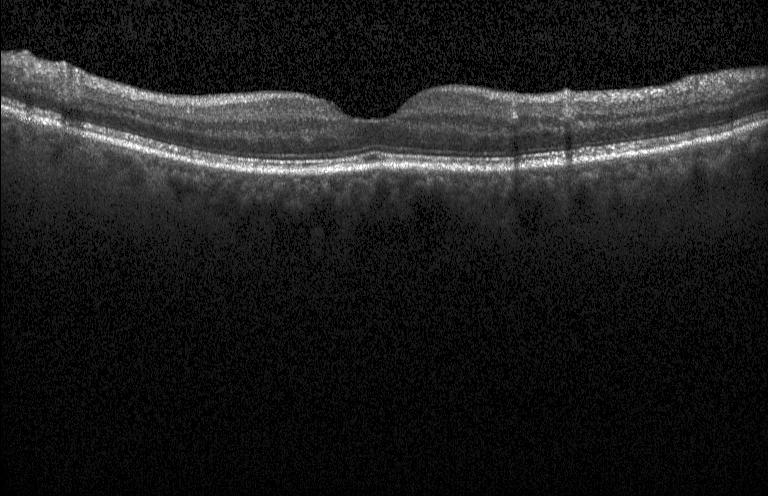
SD-OCT; optical coherence tomography scan; through the macula.
Diagnosis: no choroidal neovascularization, no diabetic macular edema, and no drusen.